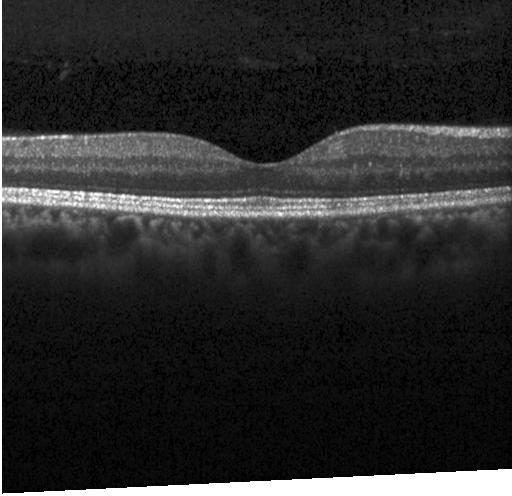
Optical coherence tomography scan · spectral-domain optical coherence tomography
OCT finding: no CNV, DME, or drusen.